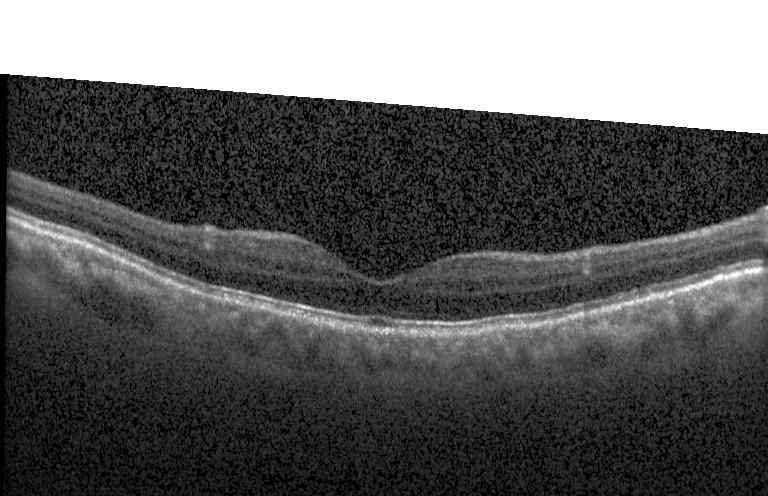
The scan shows no CNV, no DME, and no drusen.